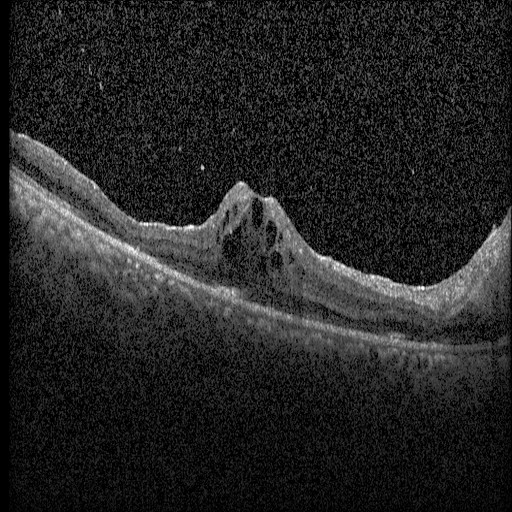

Retinal OCT cross-section, fovea-centered, Heidelberg Spectralis OCT system, spectral-domain optical coherence tomography. Diagnosis: diabetic macular edema (DME).